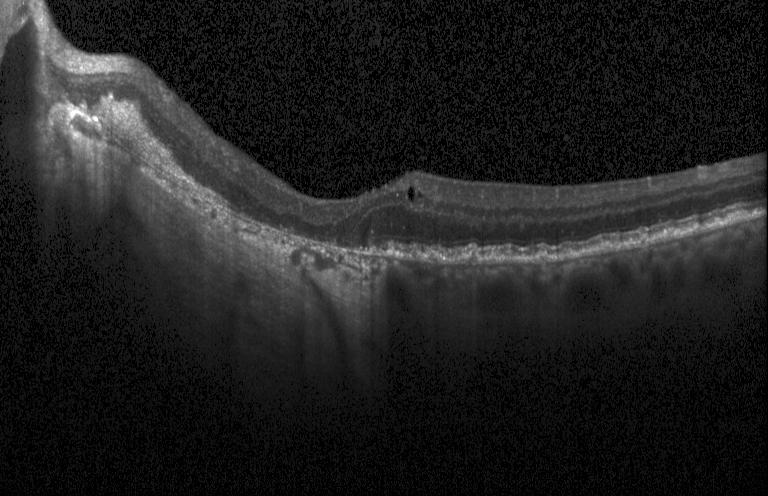
Instrument: Heidelberg Spectralis, fovea-centered, retinal OCT cross-section, spectral-domain optical coherence tomography
Dx: a choroidal neovascular membrane.